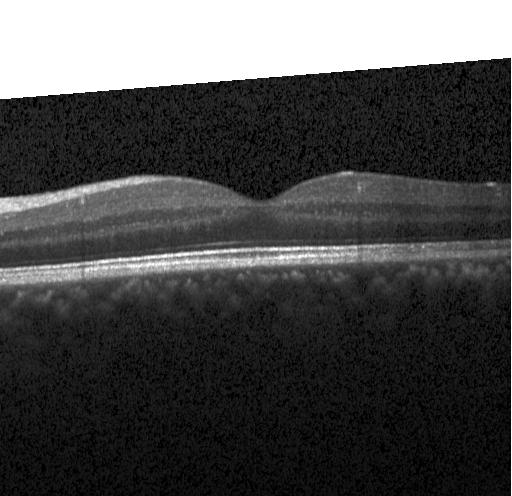
Spectral-domain OCT · centered on the fovea · retinal OCT B-scan
Diagnosis: no choroidal neovascularization, no diabetic macular edema, and no drusen.